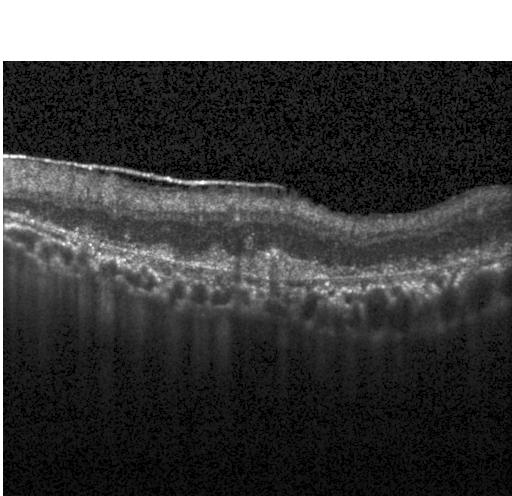

Macular OCT demonstrating a choroidal neovascular membrane.